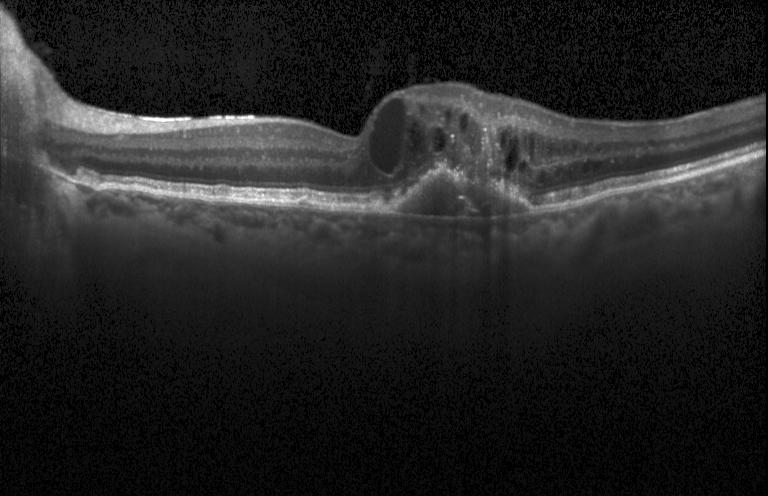

Diagnosis: a choroidal neovascular membrane.